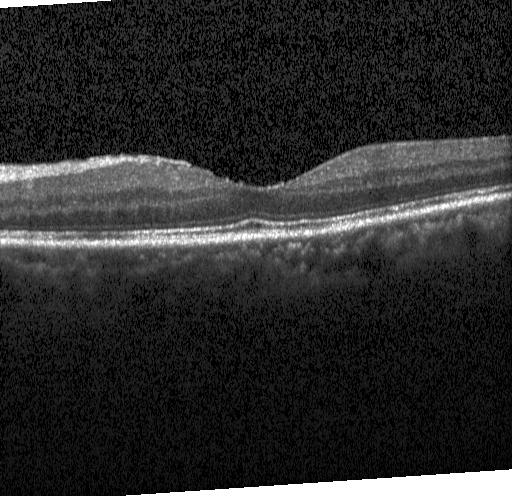

Impression: neither CNV, DME, nor drusen.